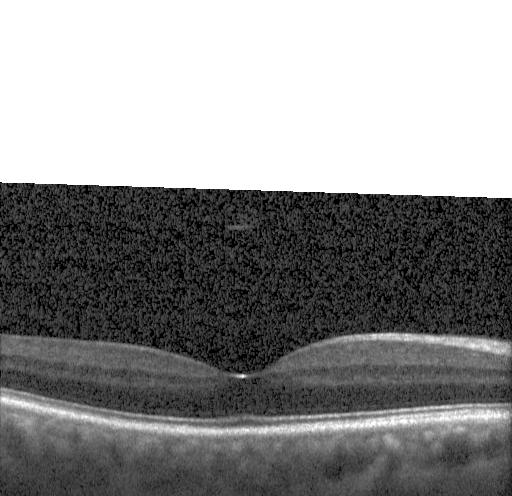
Spectral-domain OCT; retinal OCT B-scan. Assessment: no choroidal neovascularization, no diabetic macular edema, and no drusen.